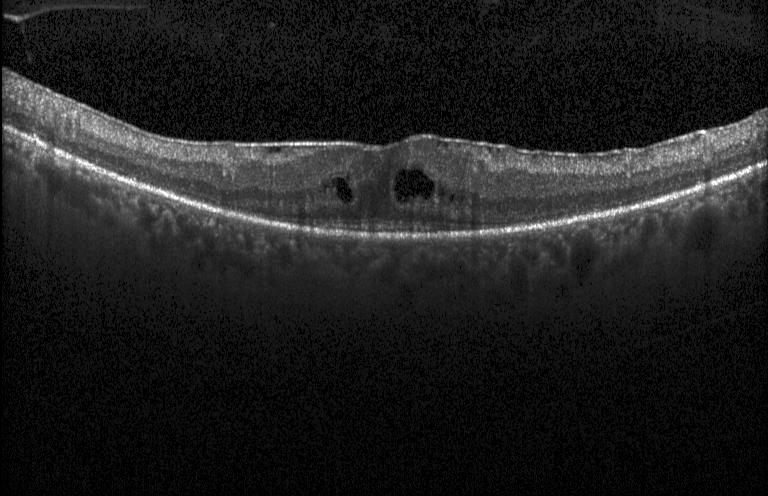
Optical coherence tomography B-scan — Assessment: diabetic macular edema.